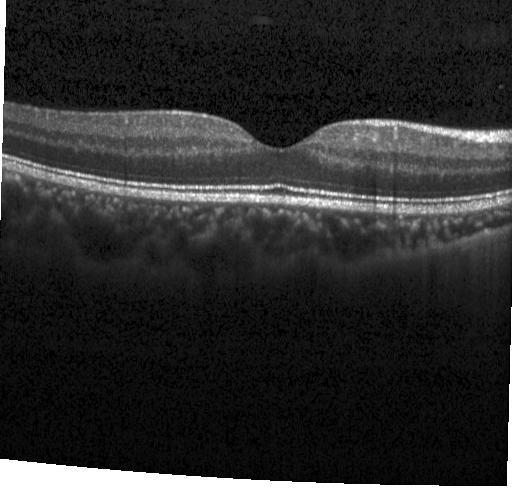 OCT B-scan; Heidelberg Spectralis OCT system
Diagnosis: no evidence of CNV, DME, or drusen.